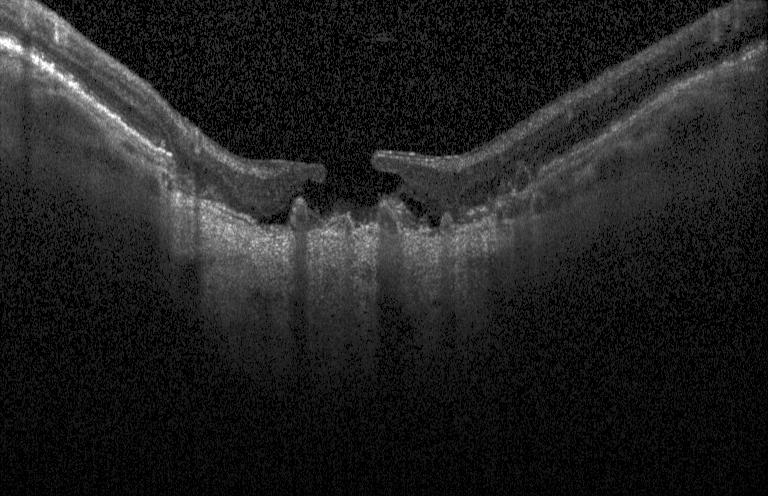

Spectral-domain optical coherence tomography · retinal OCT B-scan
Diagnosis: a choroidal neovascular membrane.